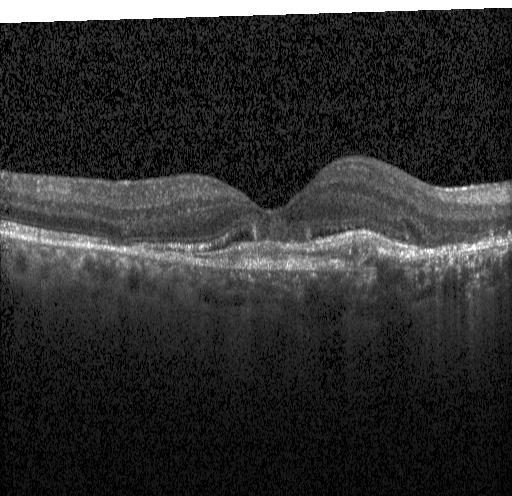

Heidelberg Spectralis · optical coherence tomography scan
Diagnosis: a choroidal neovascular membrane.